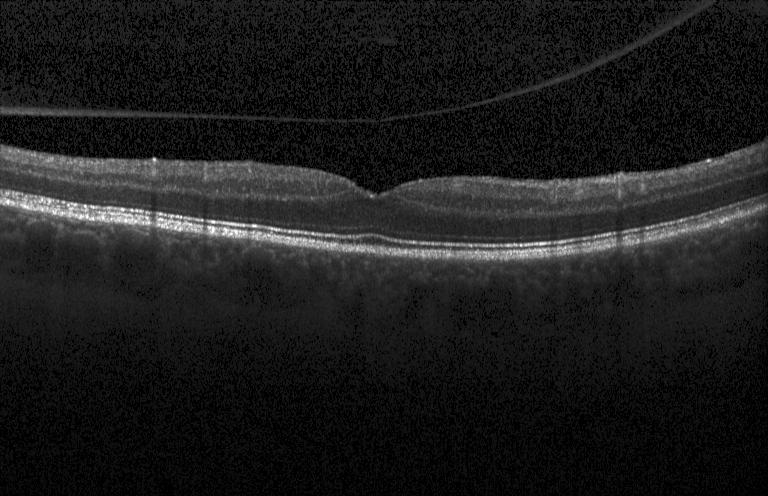
Retinal OCT B-scan.
No evidence of CNV, DME, or drusen.